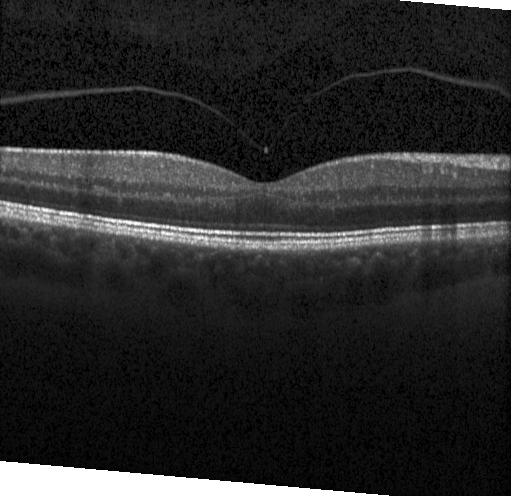 No choroidal neovascularization, diabetic macular edema, or drusen.